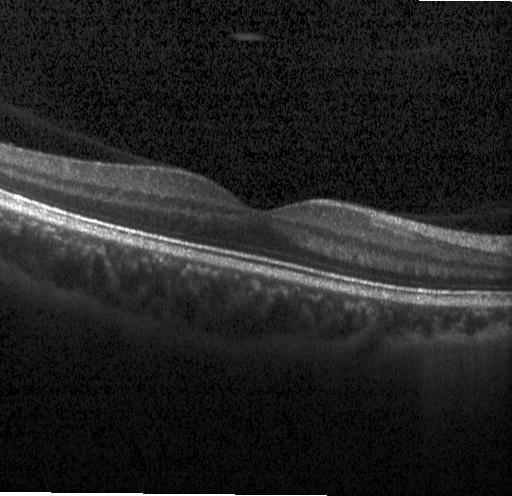

Spectral-domain OCT B-scan: no CNV, DME, or drusen.